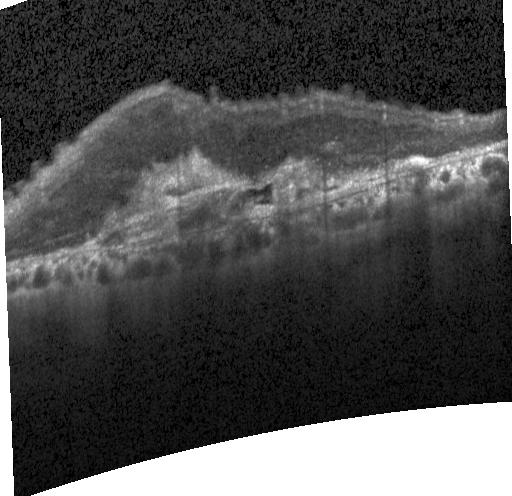
Diagnosis: choroidal neovascularization.